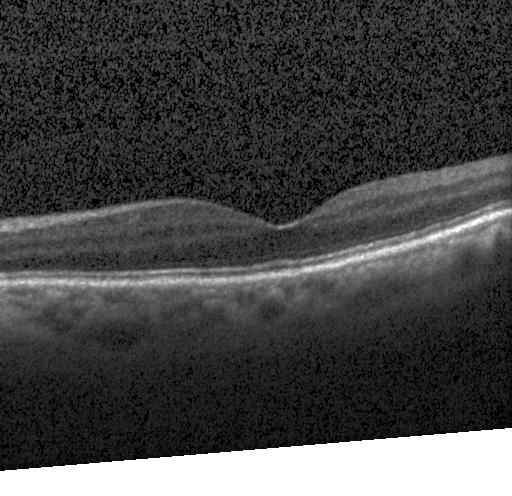
Centered on the fovea. OCT line scan
Diagnosis: no choroidal neovascularization, diabetic macular edema, or drusen.